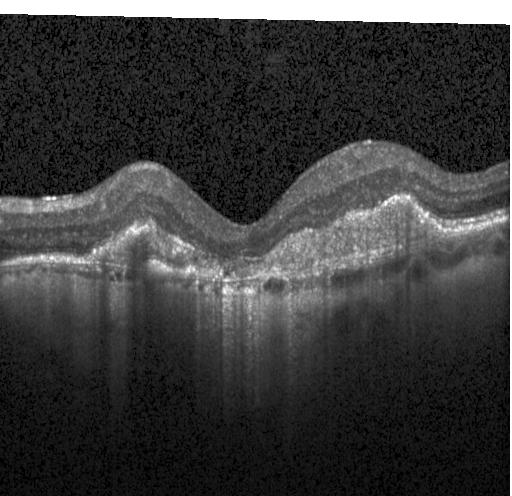

Retinal OCT cross-section showing choroidal neovascularization.